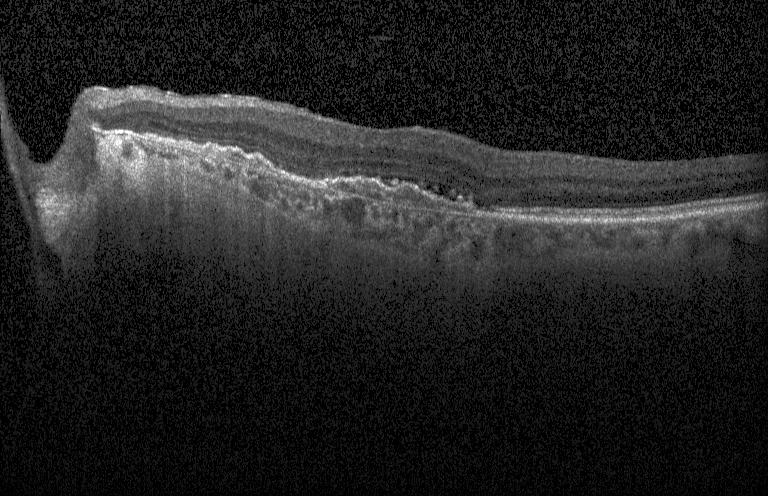
Retinal OCT cross-section · instrument: Heidelberg Spectralis. Diagnosis: a choroidal neovascular membrane.